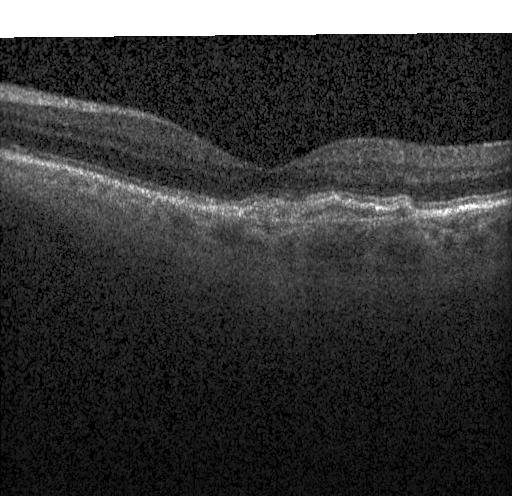
Optical coherence tomography scan.
CNV.